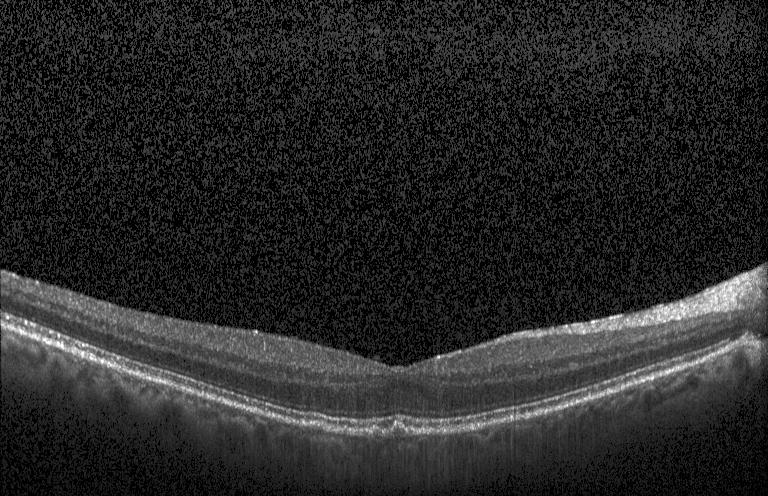
Diagnosis: drusen.